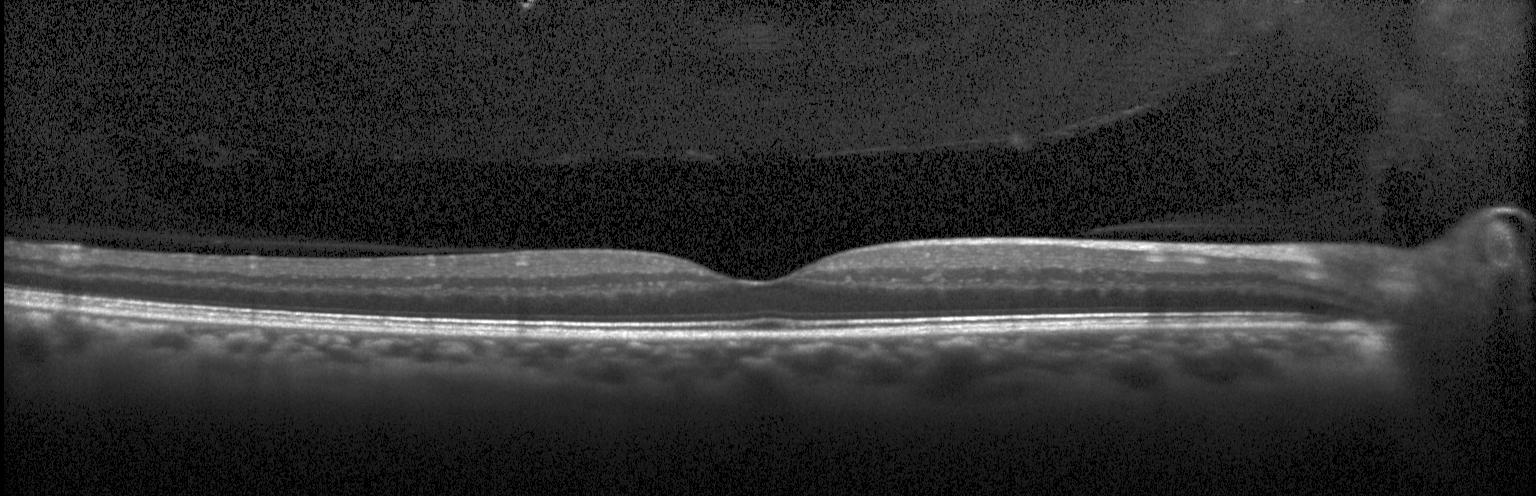
OCT B-scan. The scan shows no CNV, DME, or drusen.